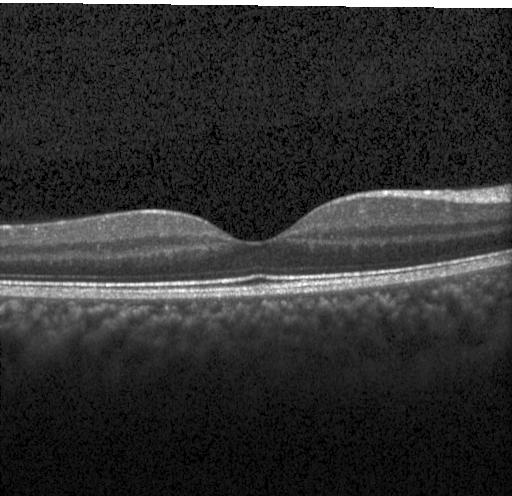
SD-OCT. Retinal OCT B-scan
This B-scan demonstrates no choroidal neovascularization, diabetic macular edema, or drusen.